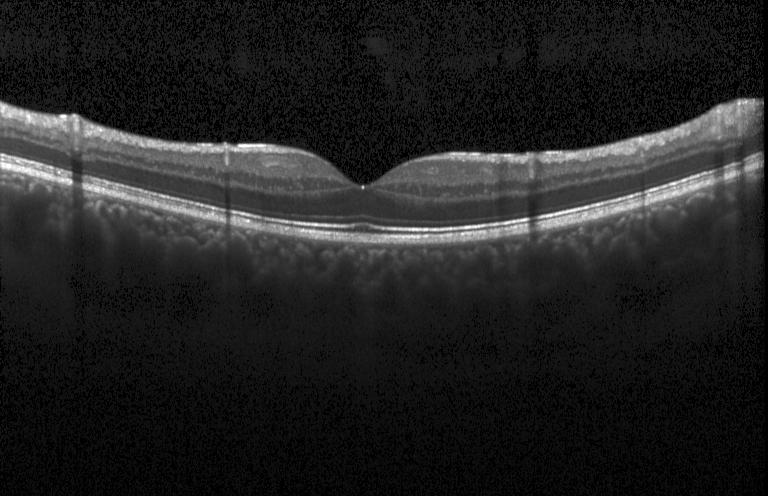
Finding: no choroidal neovascularization, no diabetic macular edema, and no drusen.